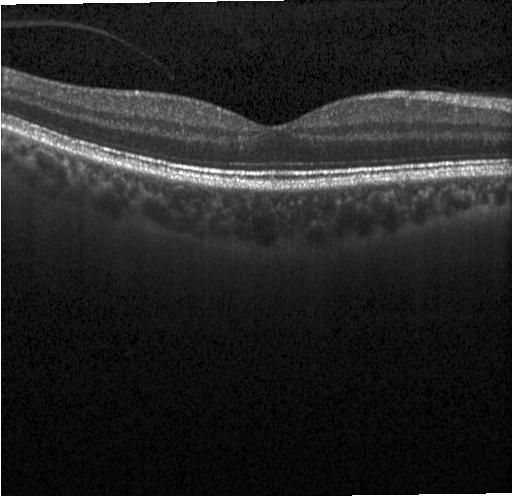

OCT B-scan; instrument: Heidelberg Spectralis — Diagnosis: no evidence of CNV, DME, or drusen.